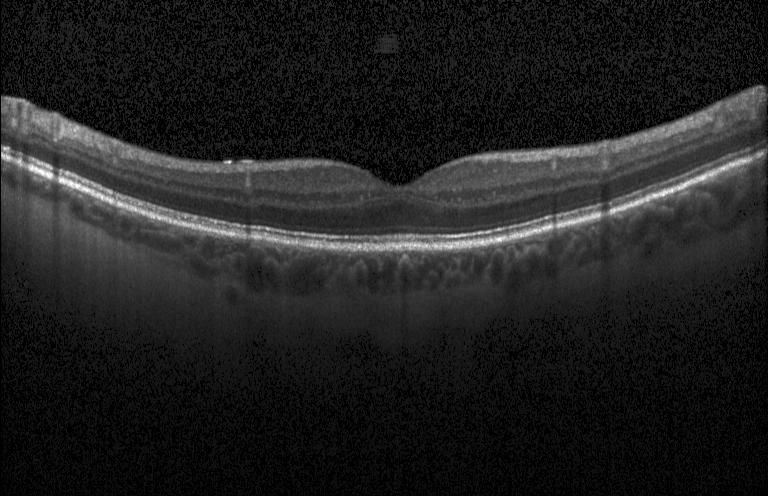

The scan shows no evidence of CNV, DME, or drusen.